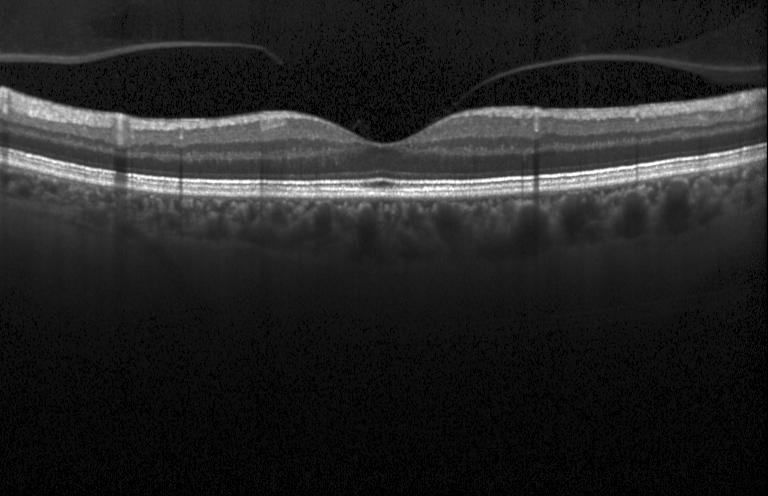
Retinal OCT cross-section · acquired on a Heidelberg Spectralis — No evidence of CNV, DME, or drusen.